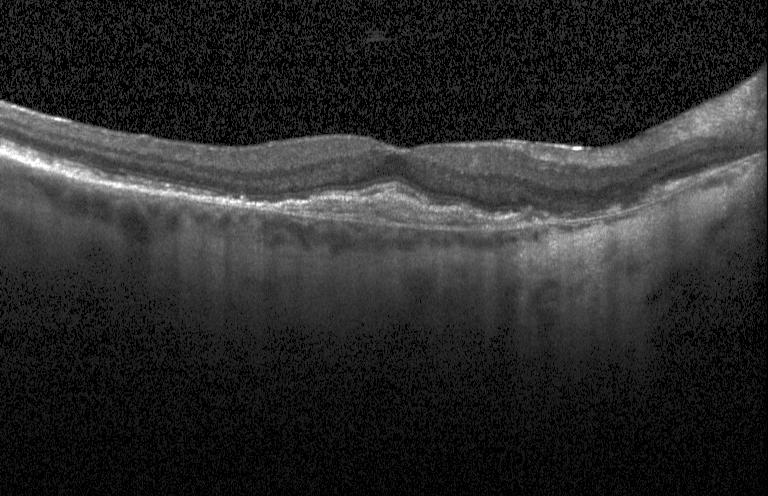 Finding: choroidal neovascularization.